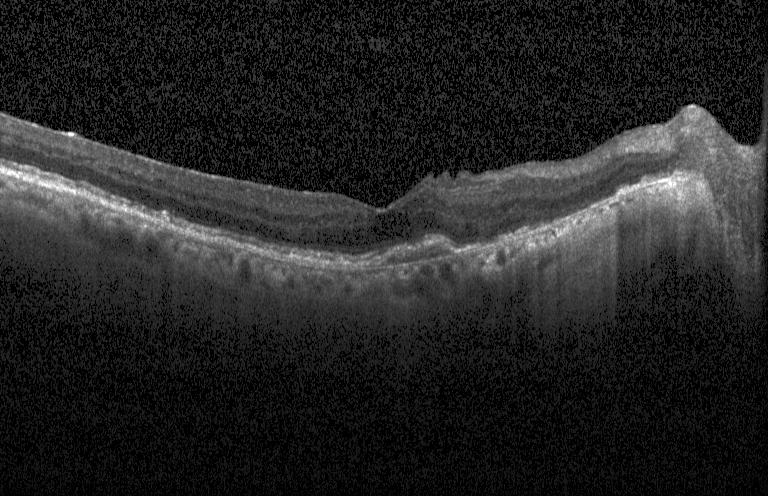
Through the macula, optical coherence tomography B-scan, instrument: Heidelberg Spectralis, spectral-domain optical coherence tomography
The scan shows CNV.